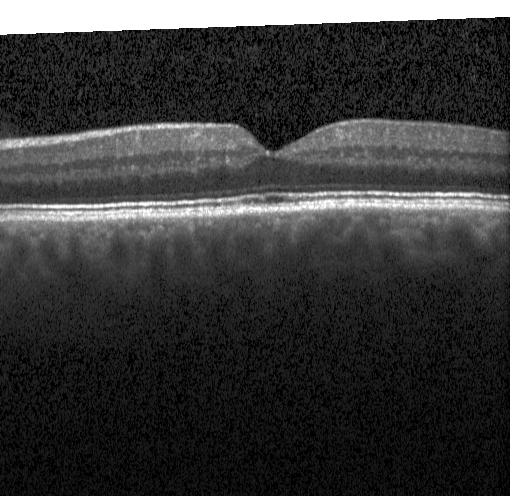 Instrument: Heidelberg Spectralis, spectral-domain optical coherence tomography, OCT B-scan
Impression: no evidence of choroidal neovascularization, diabetic macular edema, or drusen.